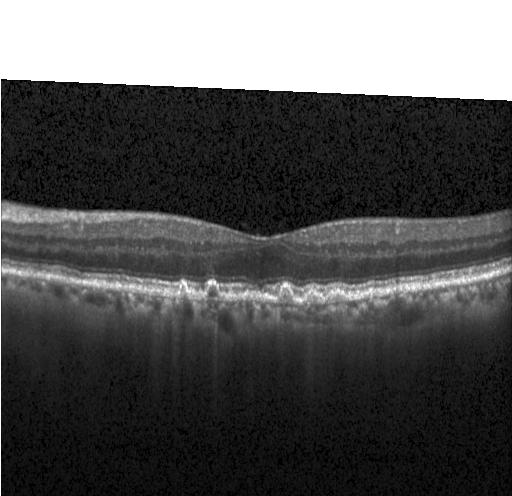 Horizontal scan through the fovea. Spectral-domain optical coherence tomography. OCT line scan
Assessment: multiple drusen.